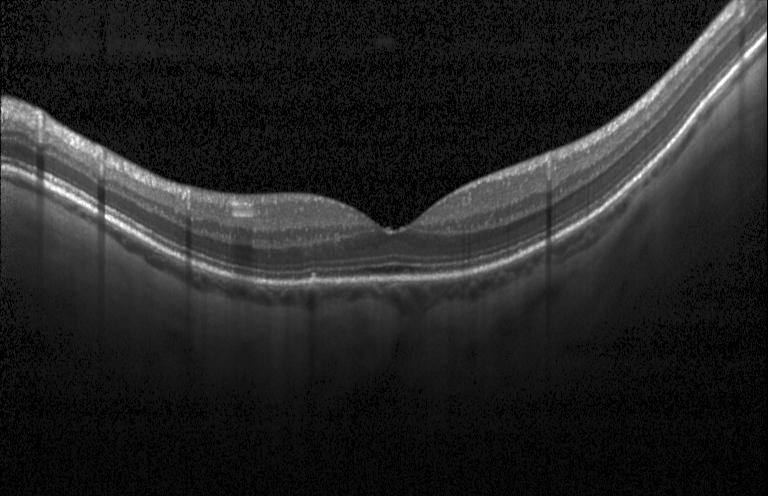
Finding: no CNV, DME, or drusen.